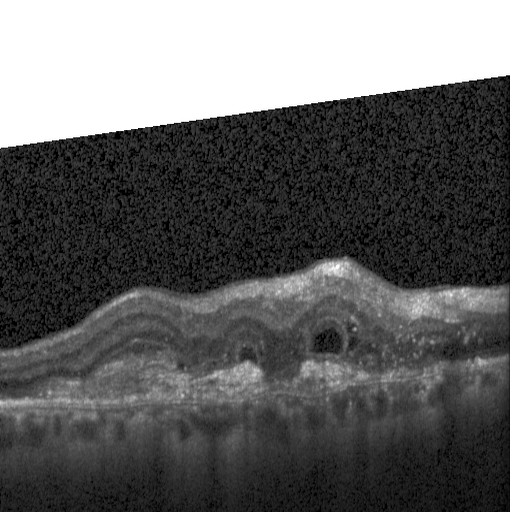

Spectral-domain optical coherence tomography. Retinal OCT B-scan. Instrument: Heidelberg Spectralis. Finding: diabetic macular edema (DME).